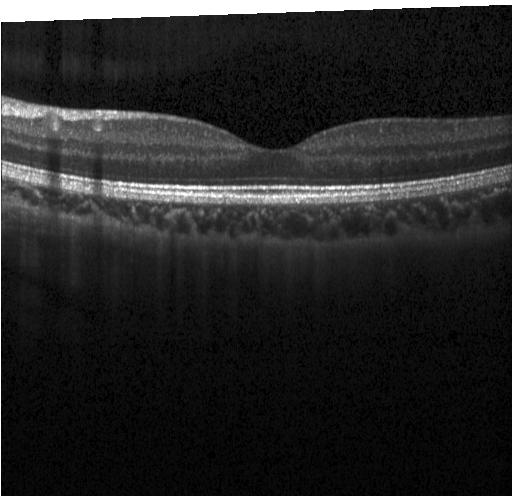
Heidelberg Spectralis OCT system, spectral-domain OCT, optical coherence tomography scan.
Finding: no choroidal neovascularization, no diabetic macular edema, and no drusen.